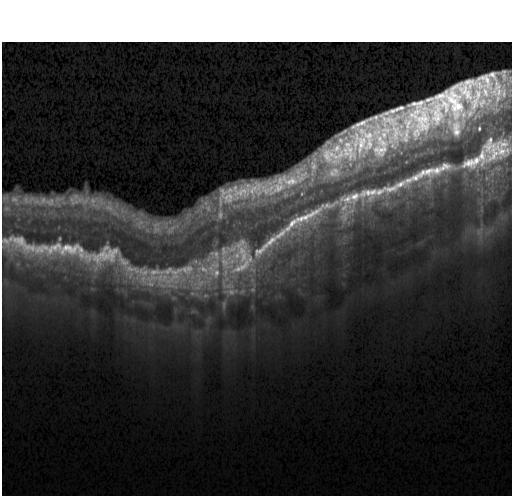
The scan shows a choroidal neovascular membrane.